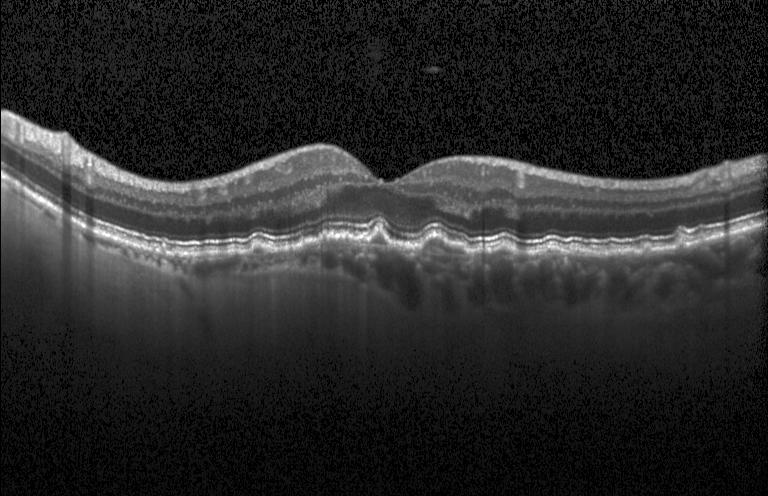

Optical coherence tomography B-scan. Acquired on a Heidelberg Spectralis. Assessment: sub-RPE drusenoid deposits.